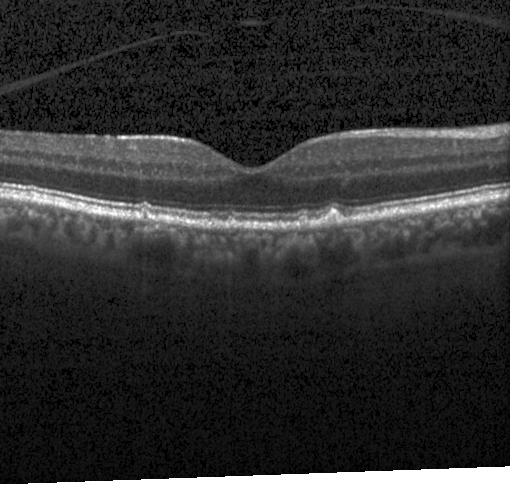

Assessment: multiple drusen.